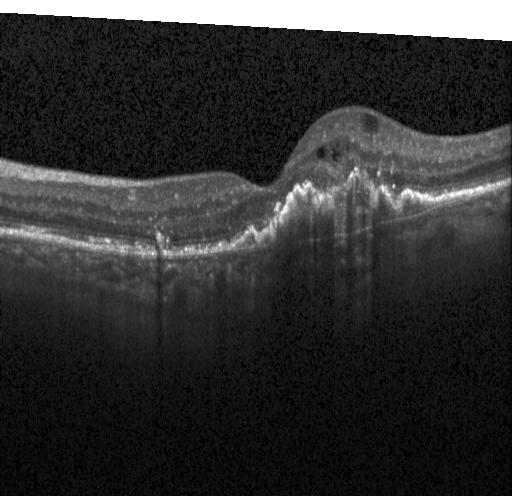 OCT B-scan showing a choroidal neovascular membrane.